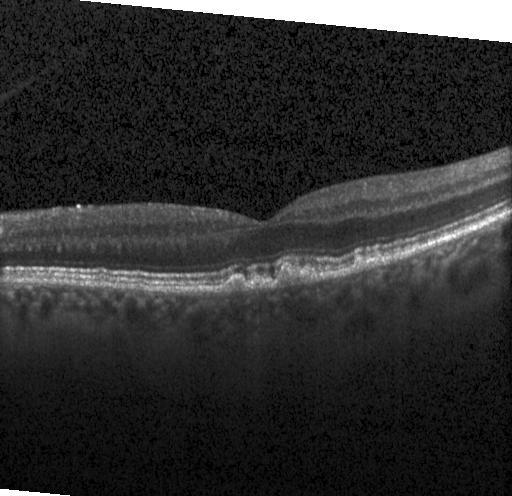

Retinal OCT cross-section; Heidelberg Spectralis; SD-OCT; fovea-centered
Finding: sub-RPE drusenoid deposits.